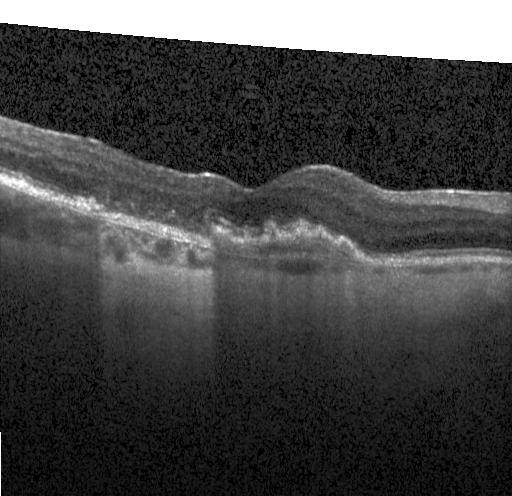
Instrument: Heidelberg Spectralis. OCT line scan — Assessment: a choroidal neovascular membrane.